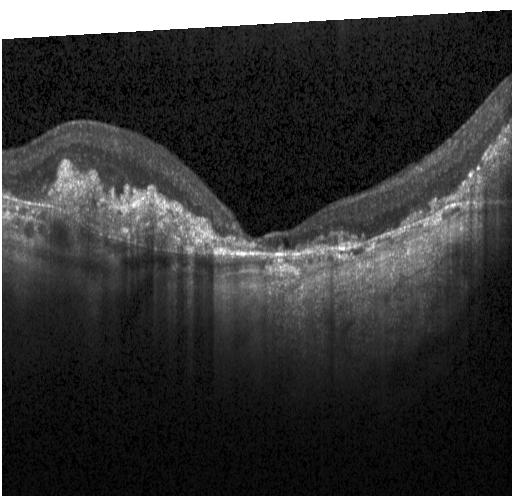 Finding: choroidal neovascularization (CNV).